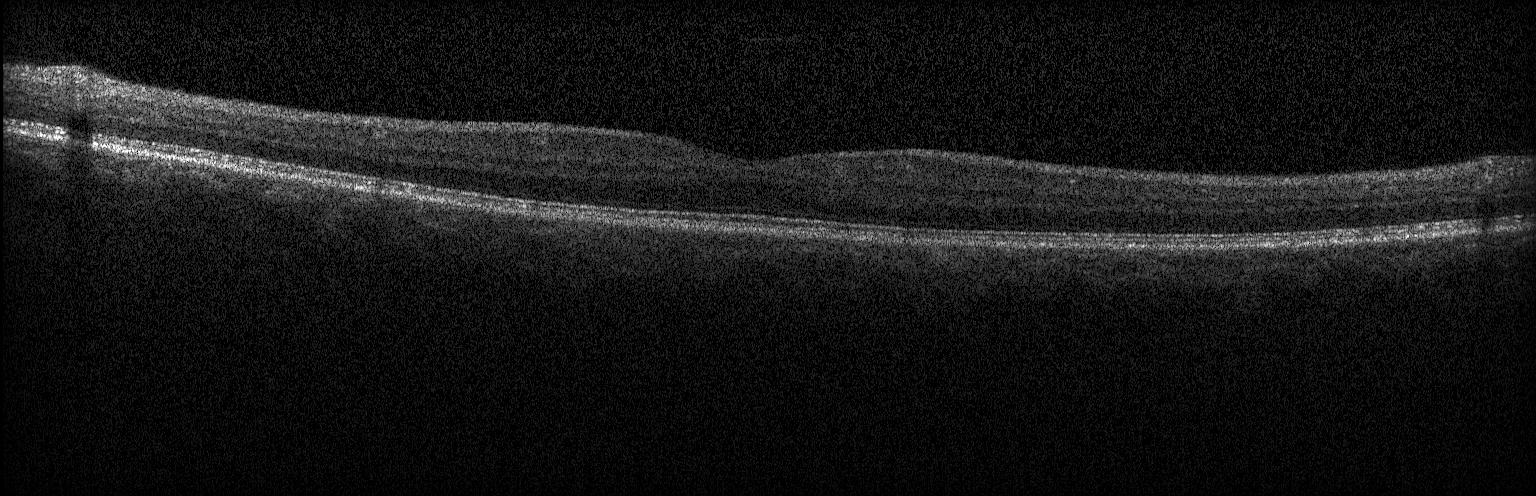

The scan shows no evidence of choroidal neovascularization, diabetic macular edema, or drusen.